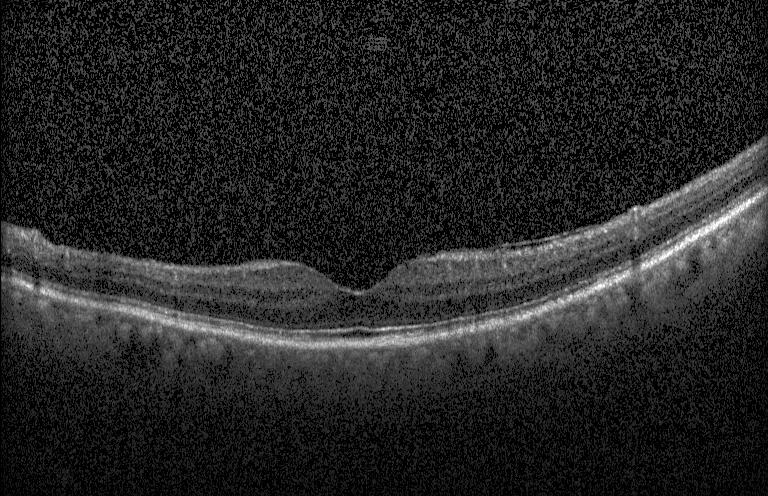

OCT scan showing no CNV, DME, or drusen.